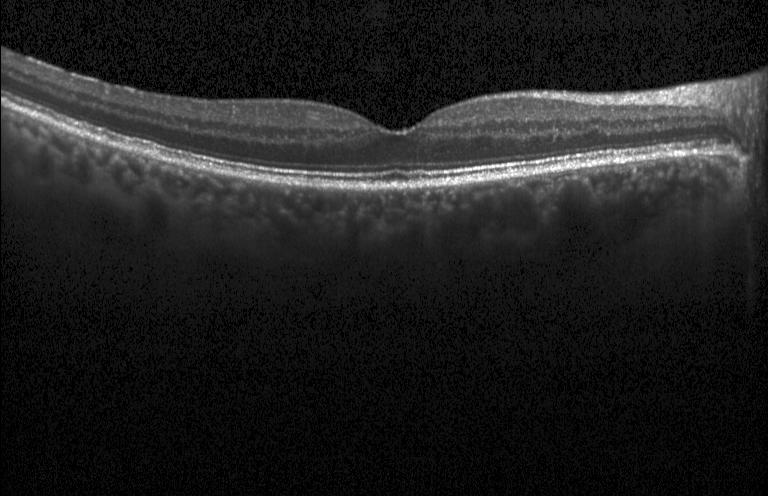

Optical coherence tomography scan. Spectral-domain optical coherence tomography. Horizontal scan through the fovea. Heidelberg Spectralis OCT system — Impression: no evidence of choroidal neovascularization, diabetic macular edema, or drusen.